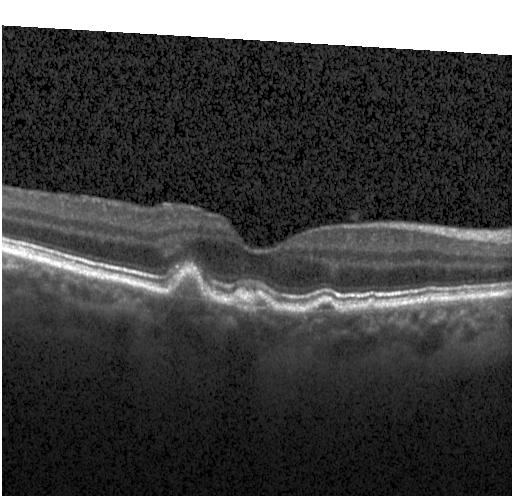
The scan shows drusen.